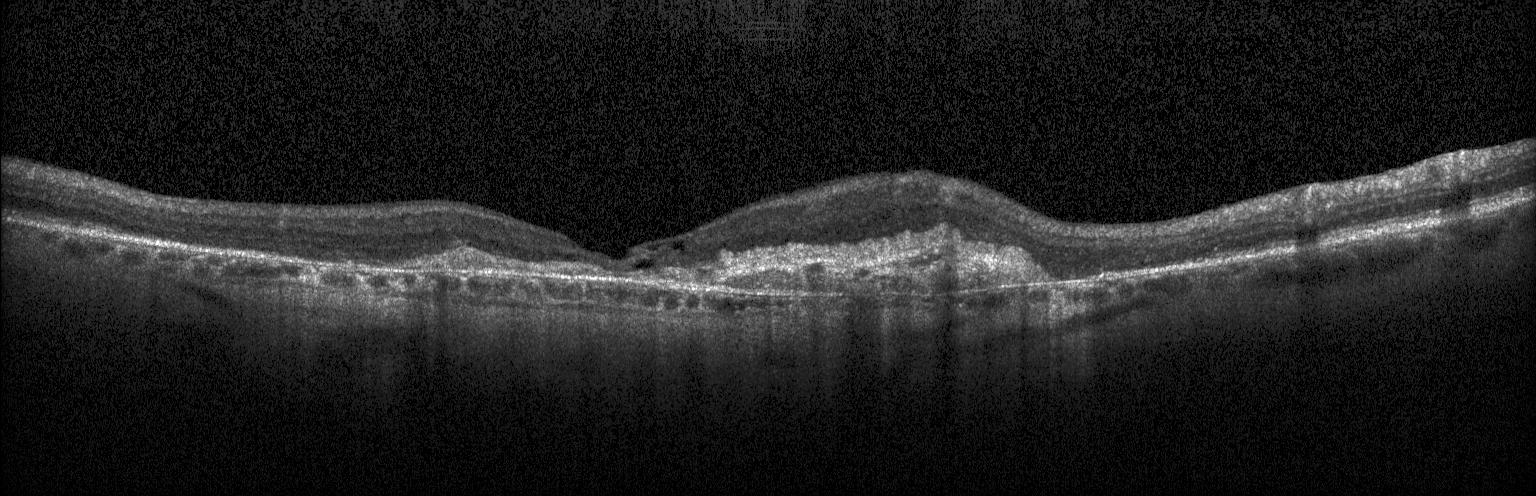
OCT scan showing CNV.